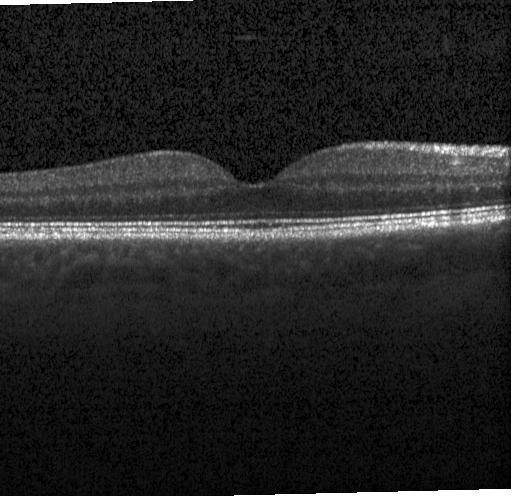 Optical coherence tomography B-scan. Through the macula. Heidelberg Spectralis OCT system. Spectral-domain OCT.
Diagnosis: no evidence of CNV, DME, or drusen.